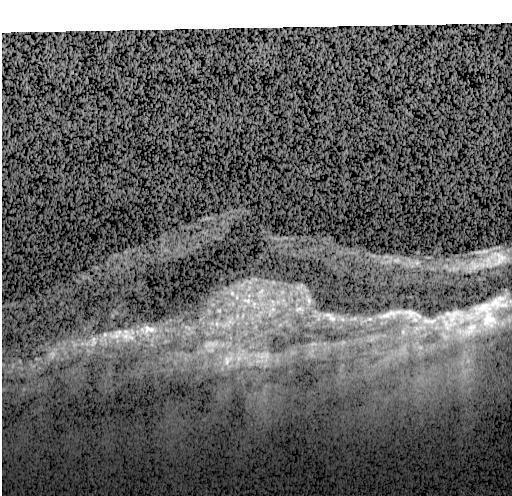 Heidelberg Spectralis. Macular scan. OCT line scan.
OCT finding: CNV.